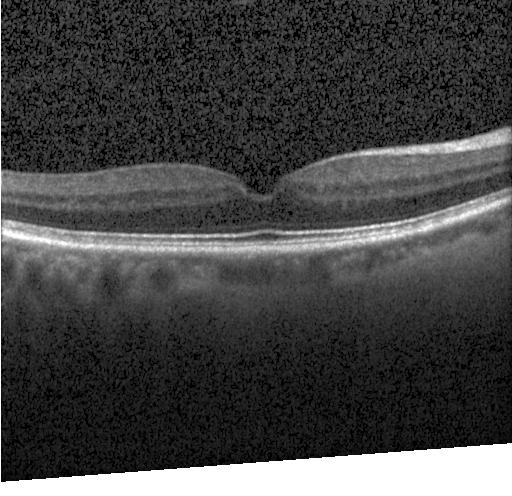

Spectral-domain optical coherence tomography, fovea-centered, instrument: Heidelberg Spectralis, retinal OCT cross-section — Diagnosis: neither choroidal neovascularization, diabetic macular edema, nor drusen.